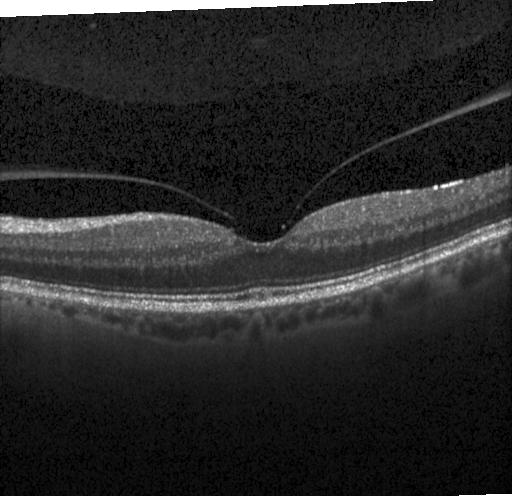
Diagnosis: no CNV, no DME, and no drusen.